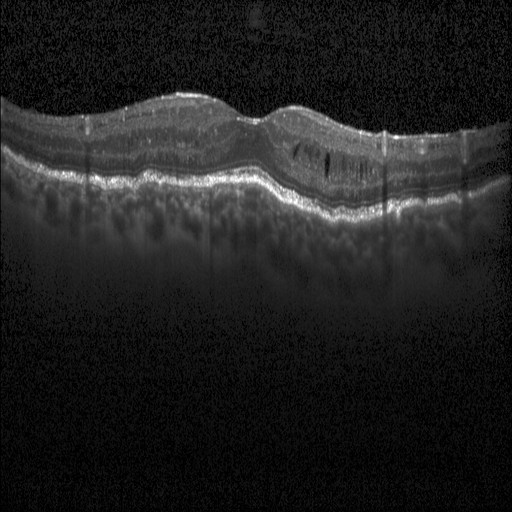 Diagnosis: diabetic macular edema.